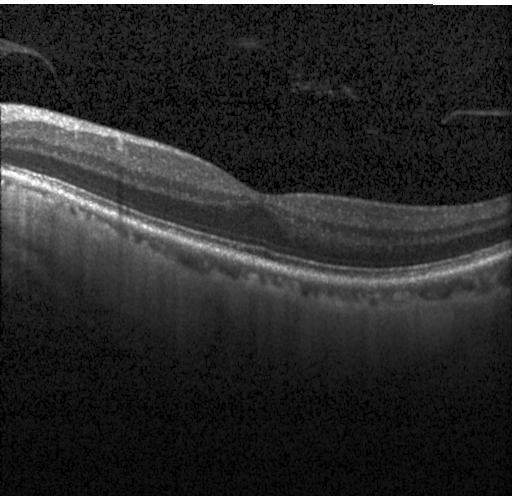
SD-OCT; horizontal scan through the fovea; retinal OCT B-scan
Diagnosis: no evidence of choroidal neovascularization, diabetic macular edema, or drusen.